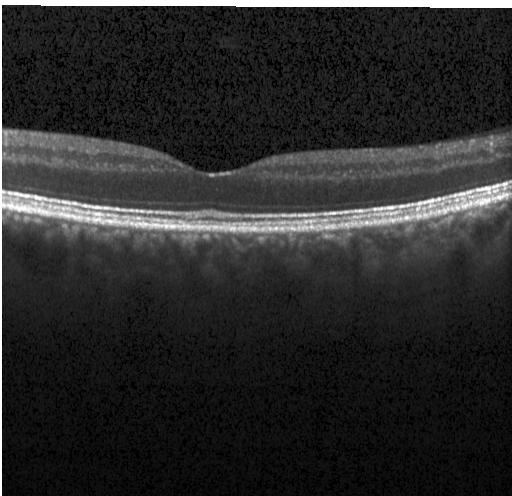
Heidelberg Spectralis OCT system, OCT line scan — The scan shows no evidence of choroidal neovascularization, diabetic macular edema, or drusen.